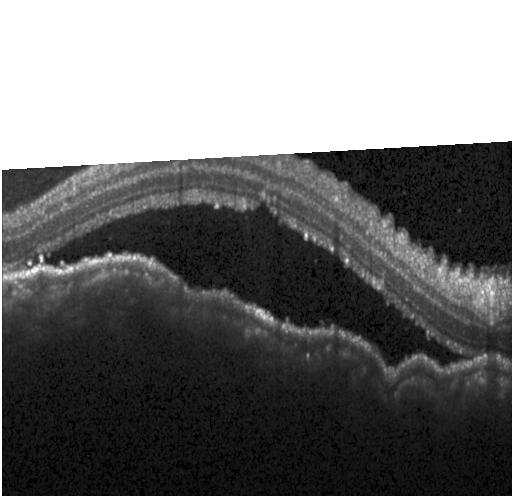 Horizontal scan through the fovea, SD-OCT, OCT B-scan — This B-scan demonstrates a choroidal neovascular membrane.